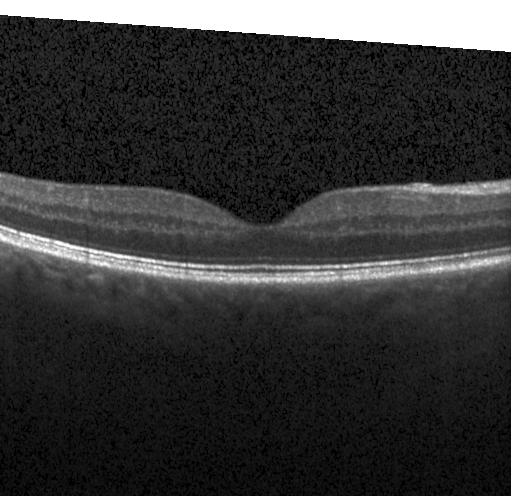 Optical coherence tomography scan
This B-scan demonstrates no choroidal neovascularization, diabetic macular edema, or drusen.